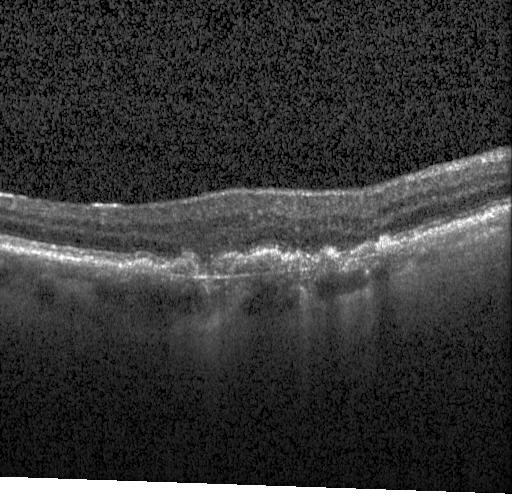
Retinal OCT B-scan; SD-OCT
Impression: CNV.